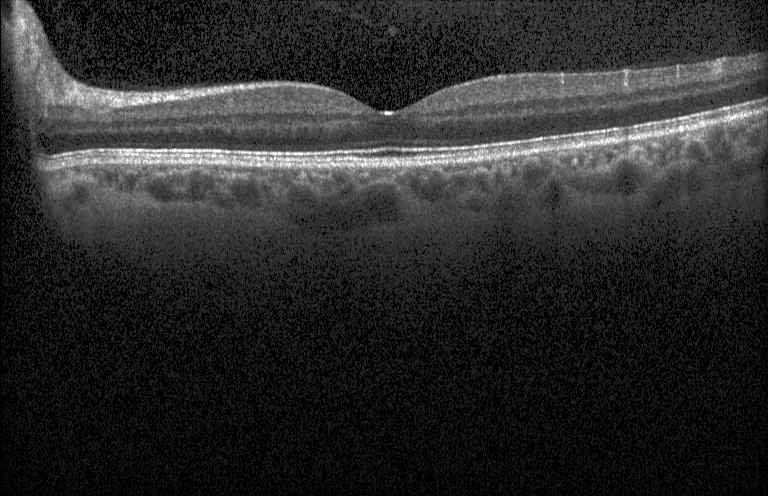
Spectral-domain OCT B-scan: no choroidal neovascularization, no diabetic macular edema, and no drusen.